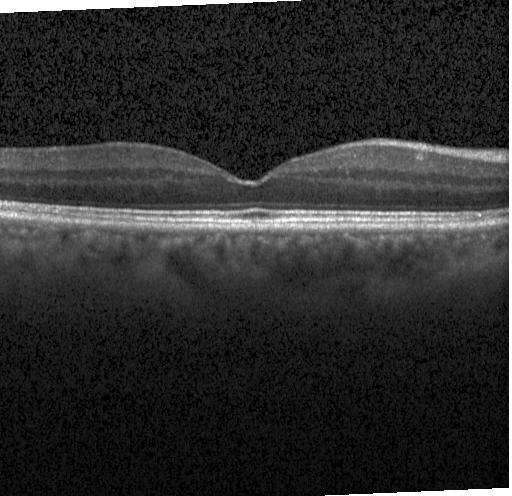
Macular scan, OCT line scan — Macular OCT: no evidence of CNV, DME, or drusen.